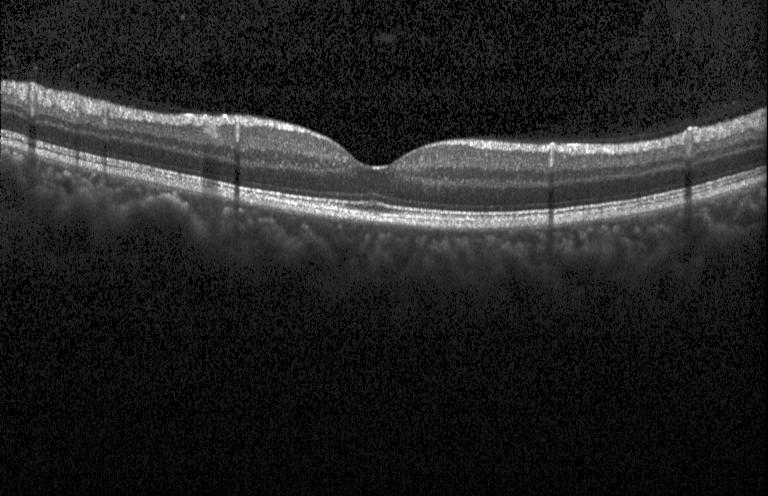

OCT B-scan showing neither CNV, DME, nor drusen.